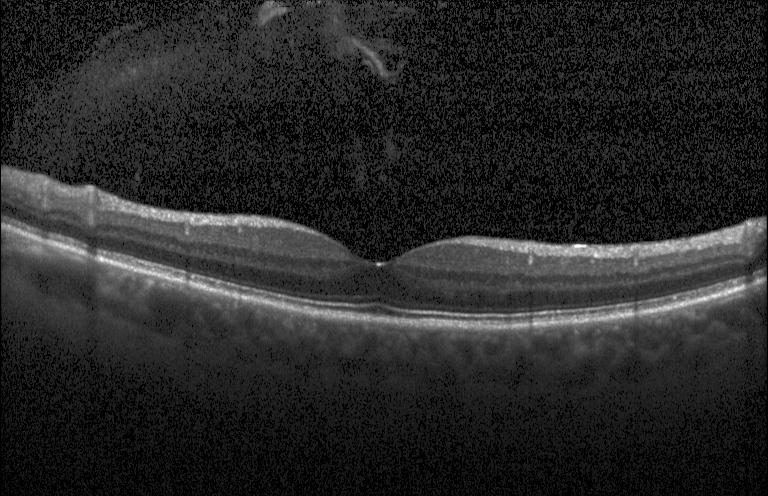
OCT finding: no evidence of CNV, DME, or drusen.